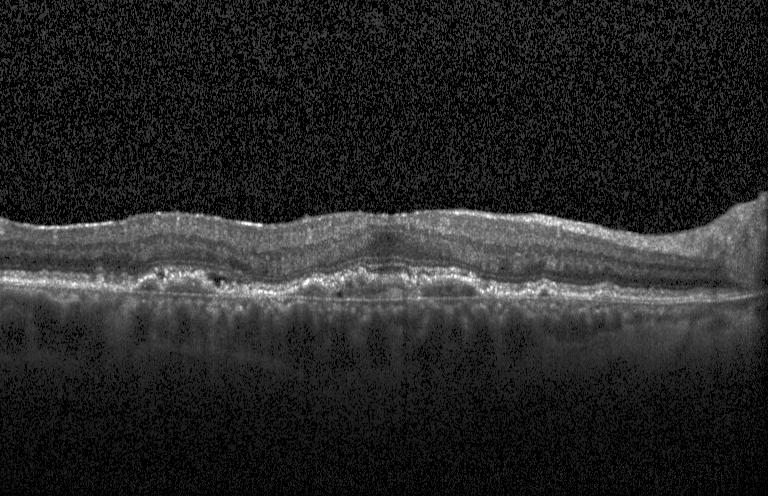 Macular OCT demonstrating choroidal neovascularization (CNV).